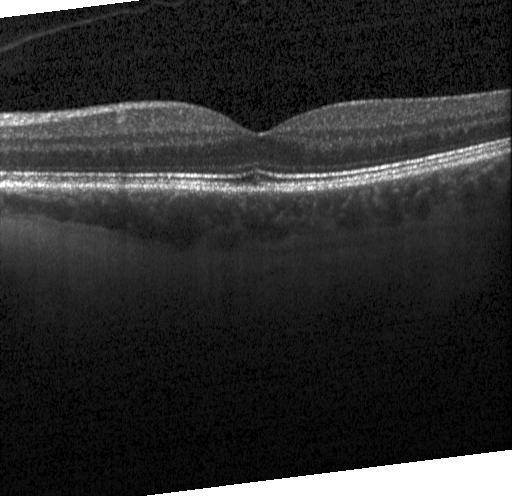 Instrument: Heidelberg Spectralis; optical coherence tomography scan. Dx: no evidence of choroidal neovascularization, diabetic macular edema, or drusen.